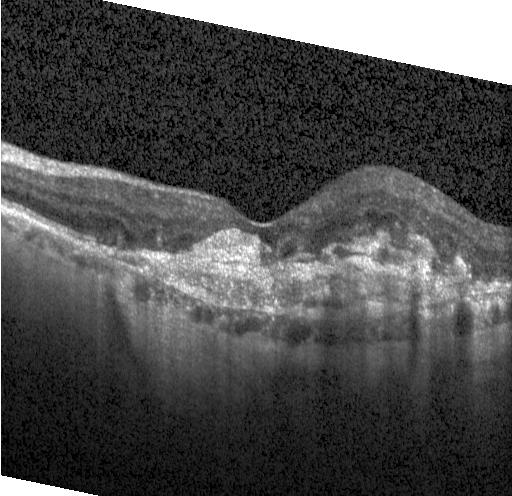
Retinal OCT B-scan · spectral-domain OCT.
Finding: choroidal neovascularization (CNV).